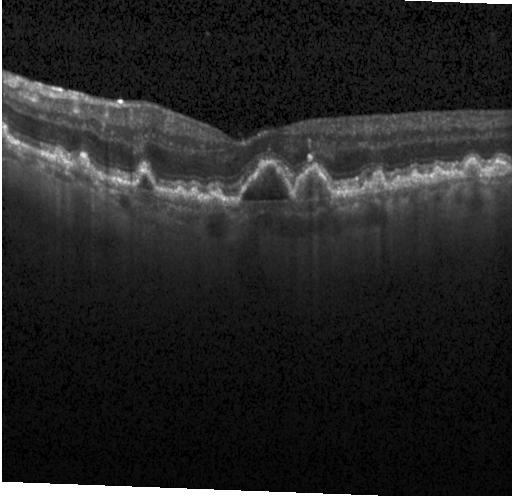
Spectral-domain OCT; centered on the fovea; OCT line scan. Diagnosis: multiple drusen.